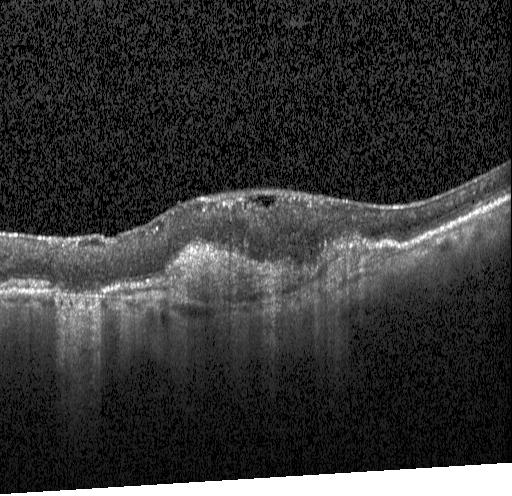
Heidelberg Spectralis. Through the macula. OCT line scan. SD-OCT. The scan shows choroidal neovascularization.